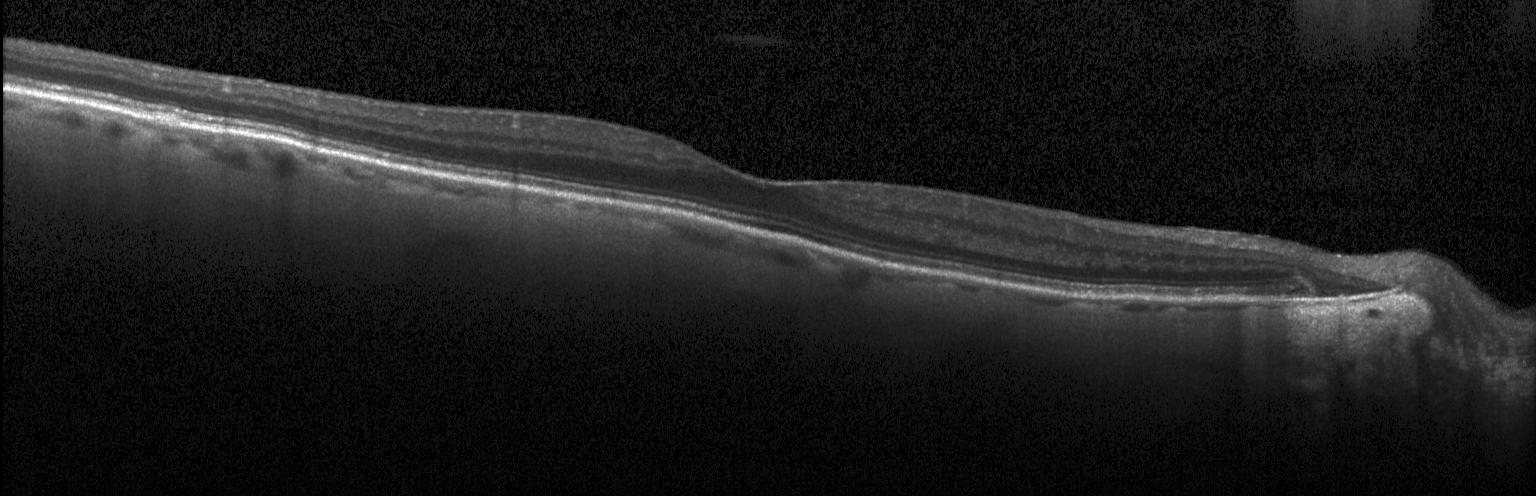

Macular OCT: neither choroidal neovascularization, diabetic macular edema, nor drusen.